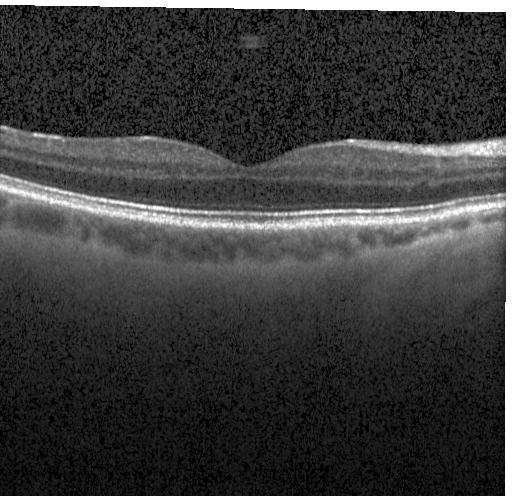
OCT finding: no CNV, no DME, and no drusen.